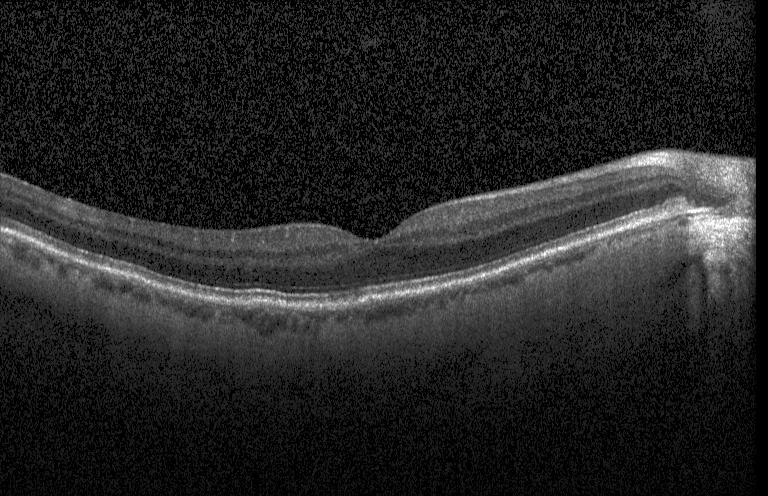

Fovea-centered · retinal OCT cross-section · acquired on a Heidelberg Spectralis — Impression: no choroidal neovascularization, diabetic macular edema, or drusen.